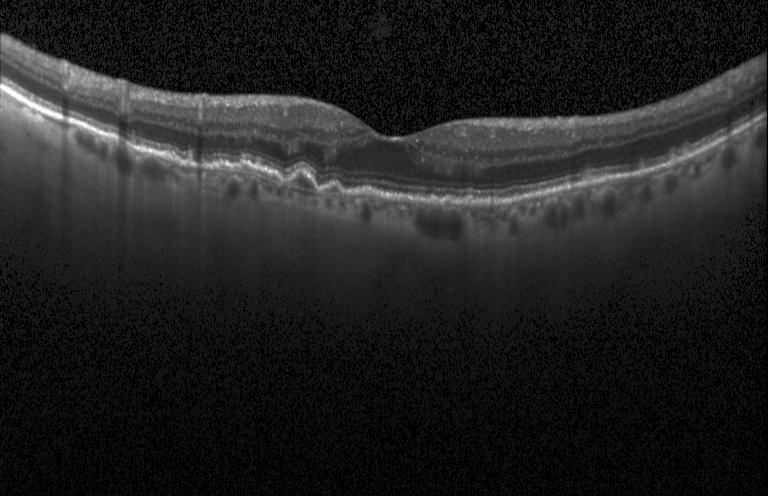

OCT line scan · instrument: Heidelberg Spectralis
Sub-RPE drusenoid deposits.